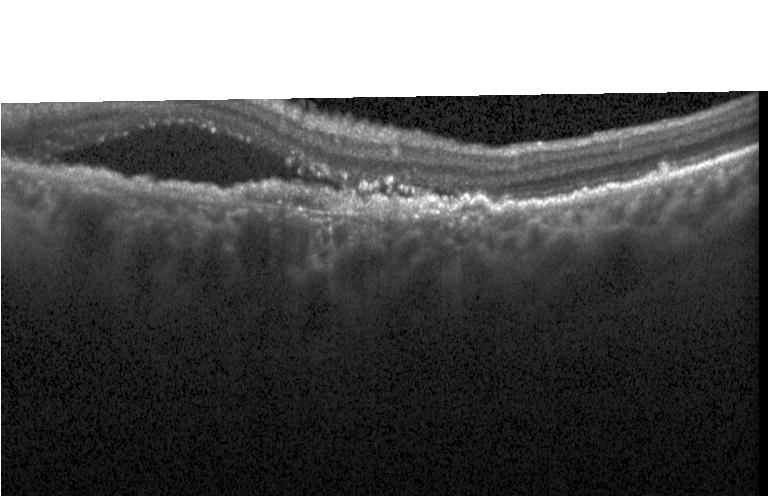

OCT line scan.
Macular OCT: choroidal neovascularization.